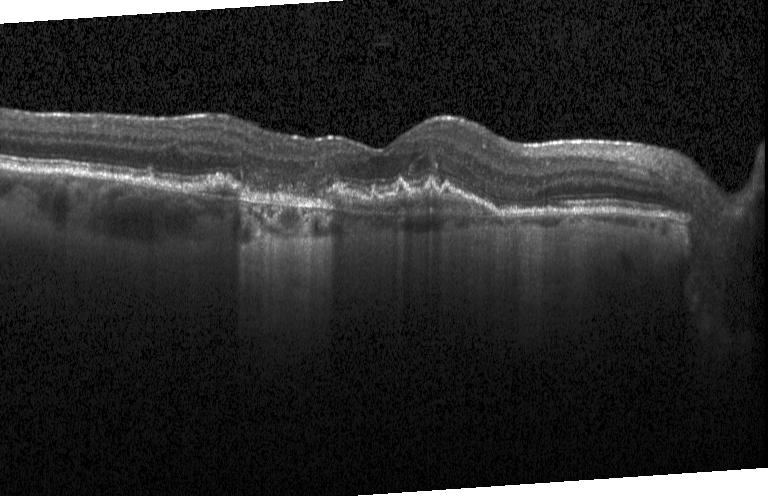 Diagnosis: choroidal neovascularization.